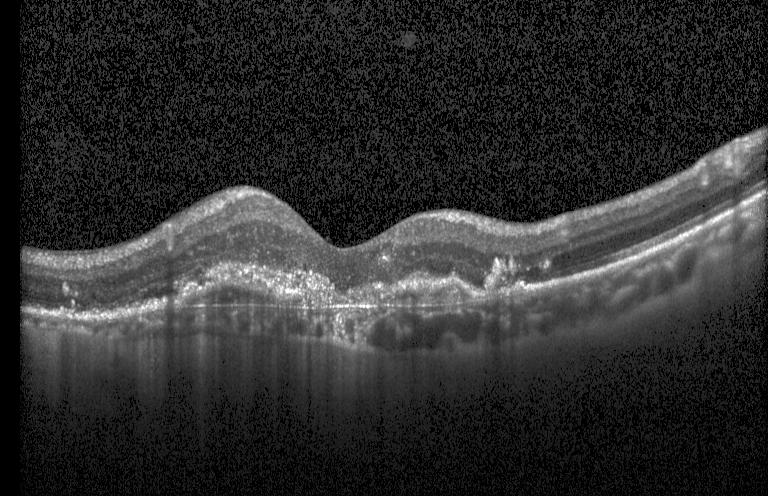 OCT B-scan showing choroidal neovascularization (CNV).